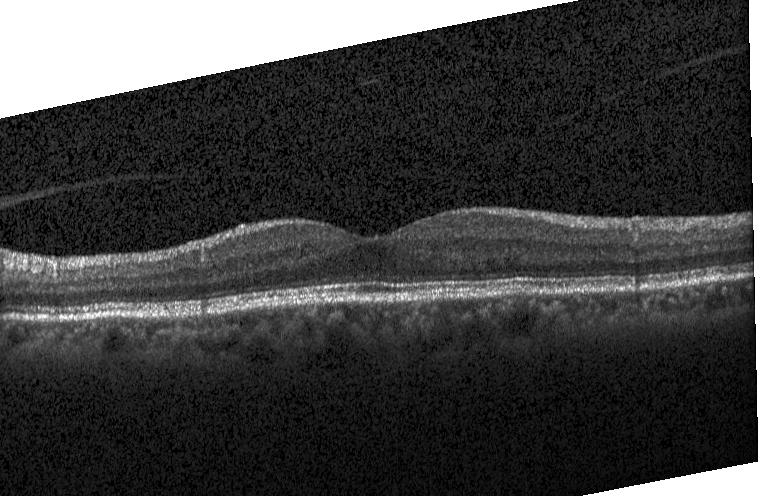
OCT finding: no CNV, no DME, and no drusen.